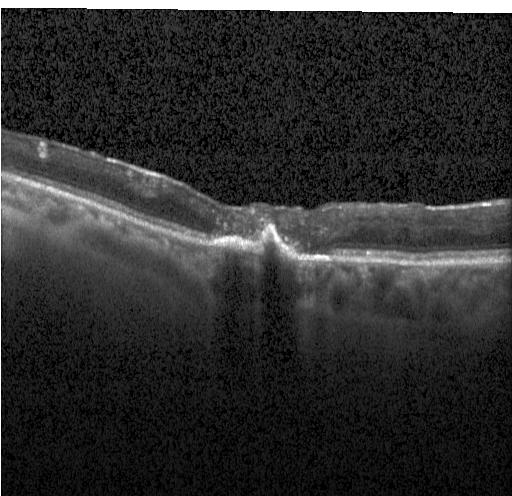
Impression: a choroidal neovascular membrane.